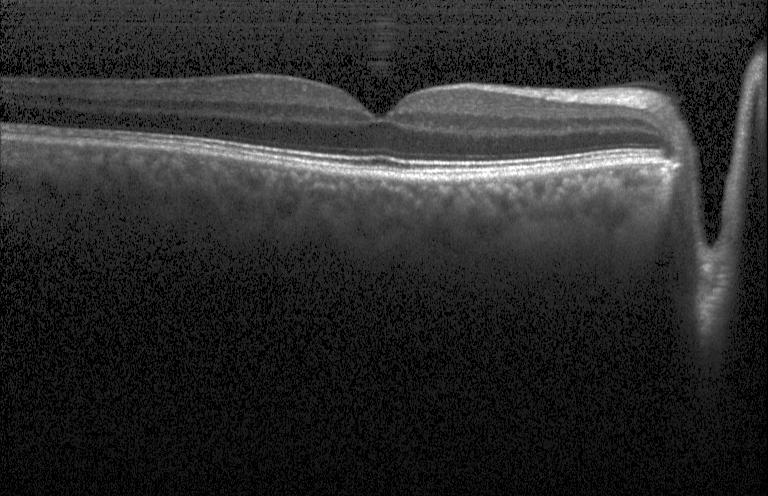 Macular OCT demonstrating no evidence of choroidal neovascularization, diabetic macular edema, or drusen.